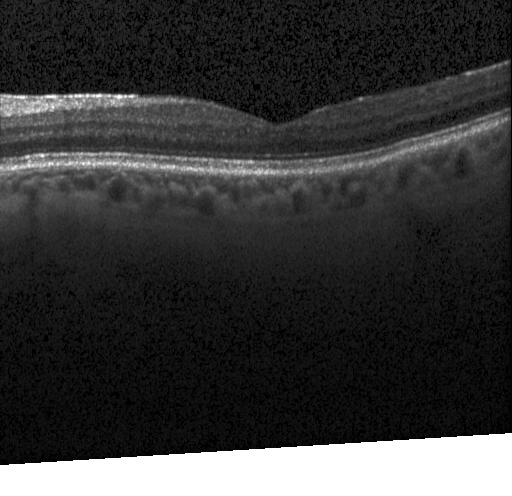

Finding: no CNV, DME, or drusen.